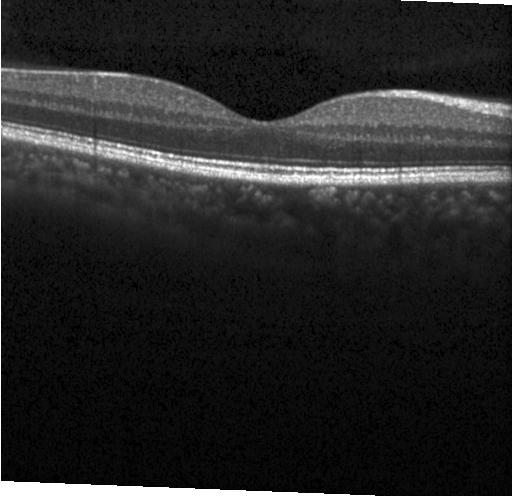 Optical coherence tomography scan
Macular OCT: neither choroidal neovascularization, diabetic macular edema, nor drusen.